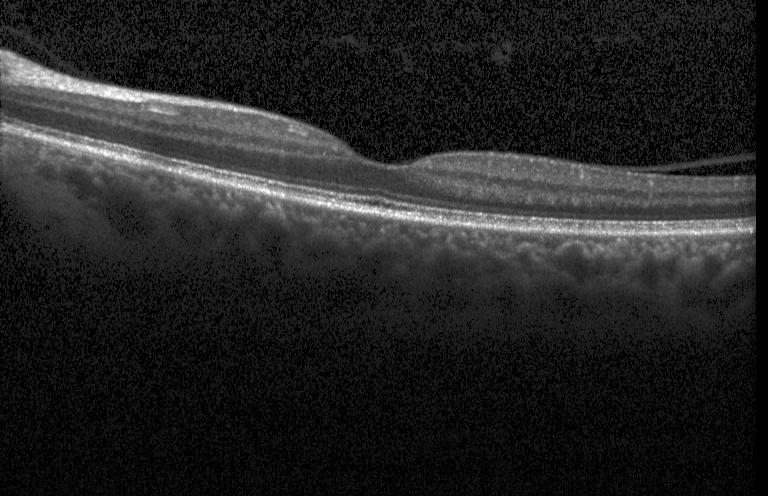
OCT scan showing no evidence of choroidal neovascularization, diabetic macular edema, or drusen.